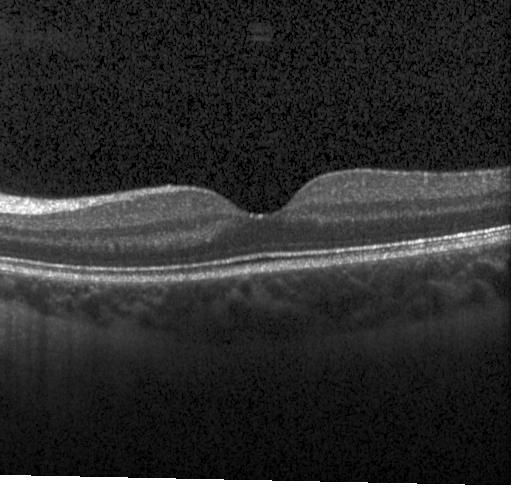 Retinal OCT B-scan; acquired on a Heidelberg Spectralis
Finding: no choroidal neovascularization, diabetic macular edema, or drusen.